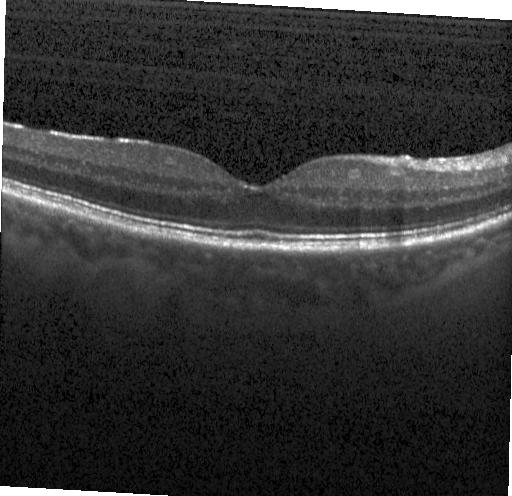

Assessment: neither choroidal neovascularization, diabetic macular edema, nor drusen.